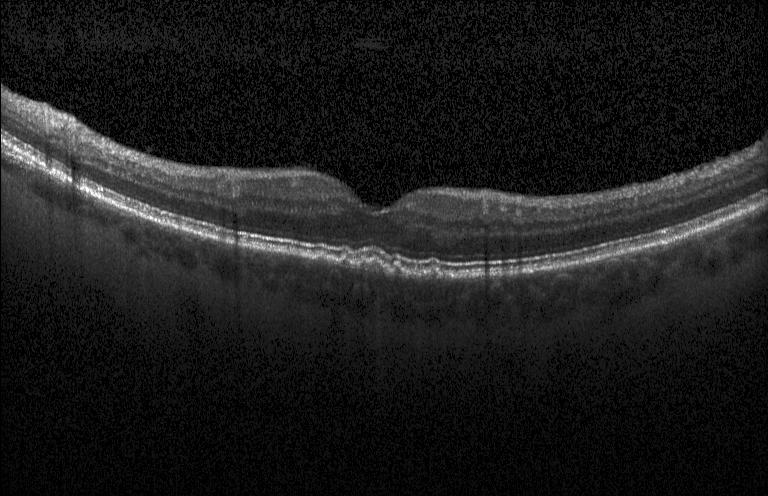
Optical coherence tomography B-scan. Heidelberg Spectralis OCT system. SD-OCT. Horizontal scan through the fovea
Diagnosis: drusen.